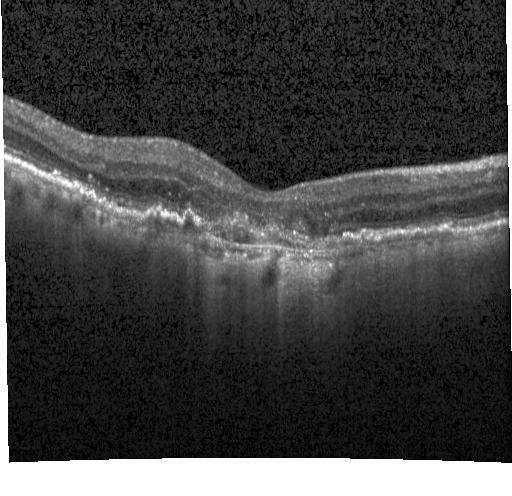
Retinal OCT cross-section; through the macula; instrument: Heidelberg Spectralis
Diagnosis: a choroidal neovascular membrane.